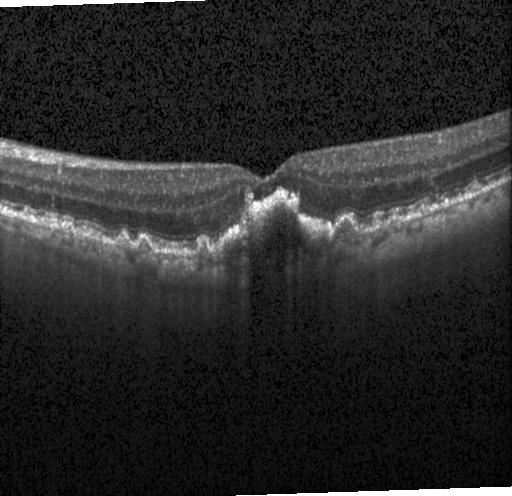

OCT scan showing a choroidal neovascular membrane.